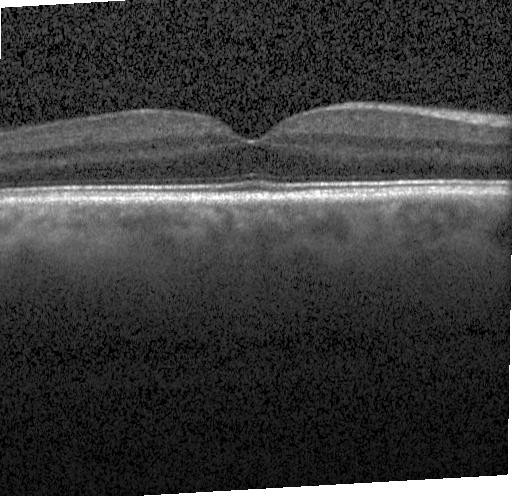
Instrument: Heidelberg Spectralis · through the macula · OCT B-scan · spectral-domain optical coherence tomography — Impression: neither choroidal neovascularization, diabetic macular edema, nor drusen.